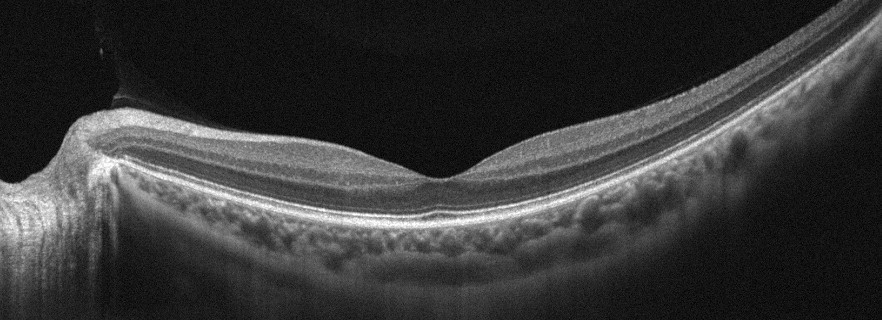 Dx: no evidence of AMD, DME, ERM, RAO, RVO, or VID.